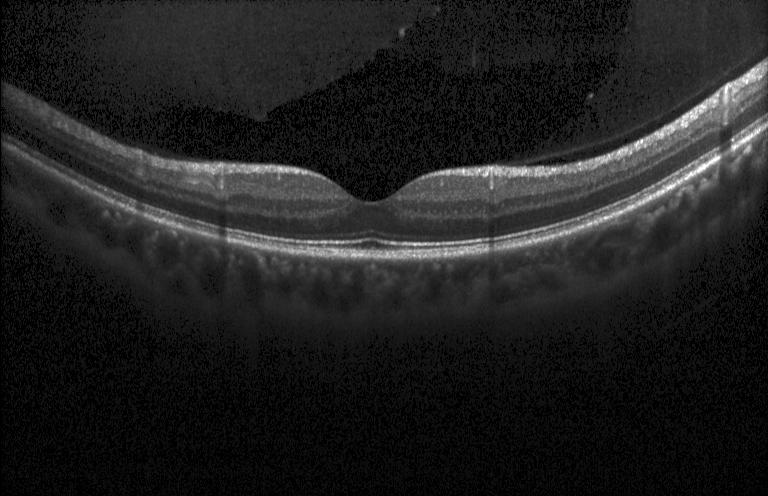

OCT B-scan showing no CNV, DME, or drusen.